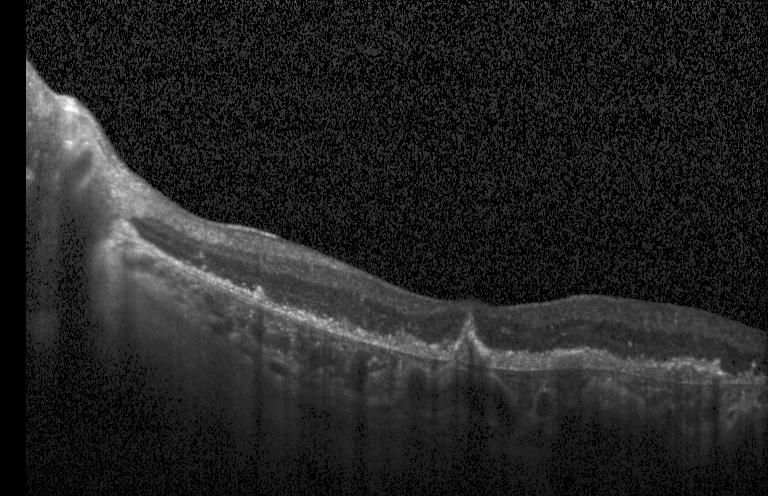
Retinal OCT B-scan; Heidelberg Spectralis OCT system; macular scan; spectral-domain OCT.
Finding: a choroidal neovascular membrane.